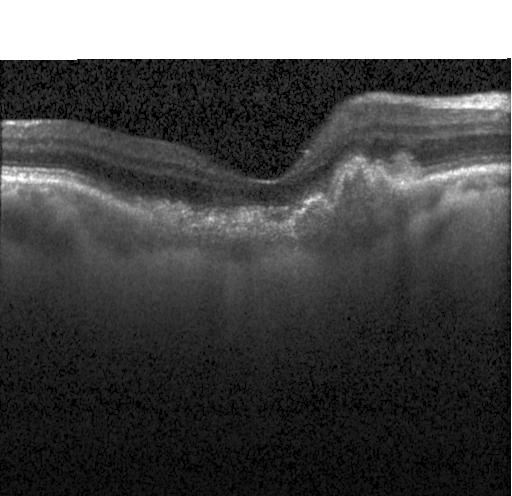
Horizontal scan through the fovea. OCT line scan — Finding: choroidal neovascularization (CNV).